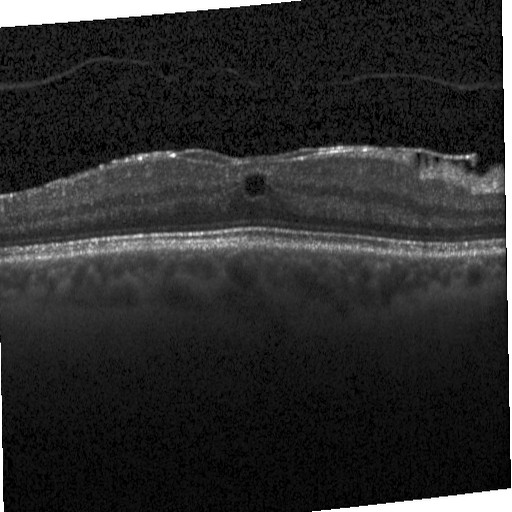 Macular OCT demonstrating diabetic macular edema (DME).